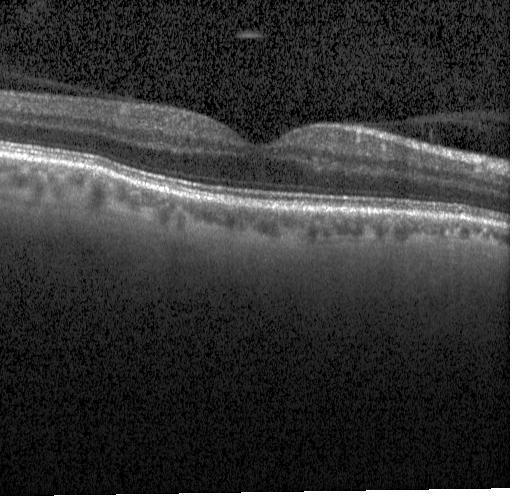

The scan shows no CNV, no DME, and no drusen.